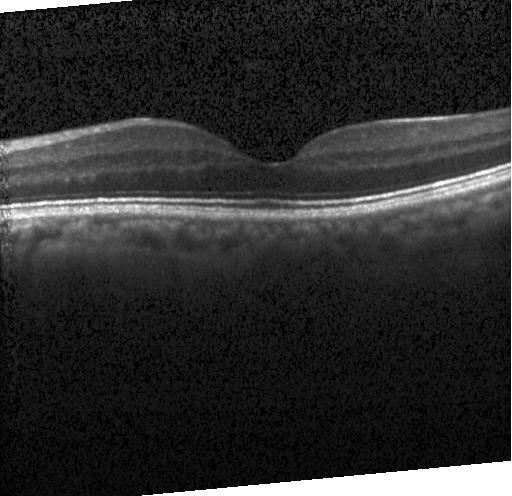 OCT B-scan · acquired on a Heidelberg Spectralis — Impression: neither choroidal neovascularization, diabetic macular edema, nor drusen.